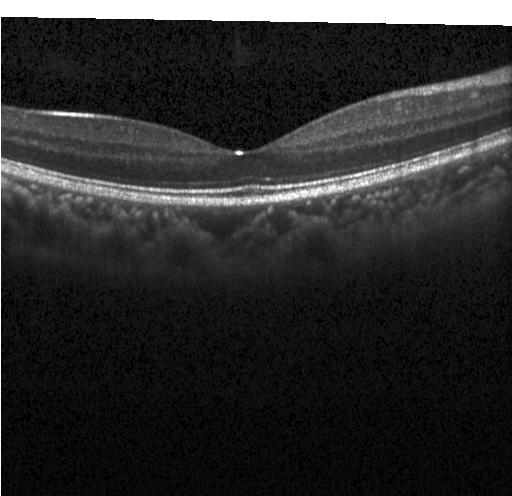 Centered on the fovea; acquired on a Heidelberg Spectralis; SD-OCT; OCT B-scan
Diagnosis: no choroidal neovascularization, no diabetic macular edema, and no drusen.